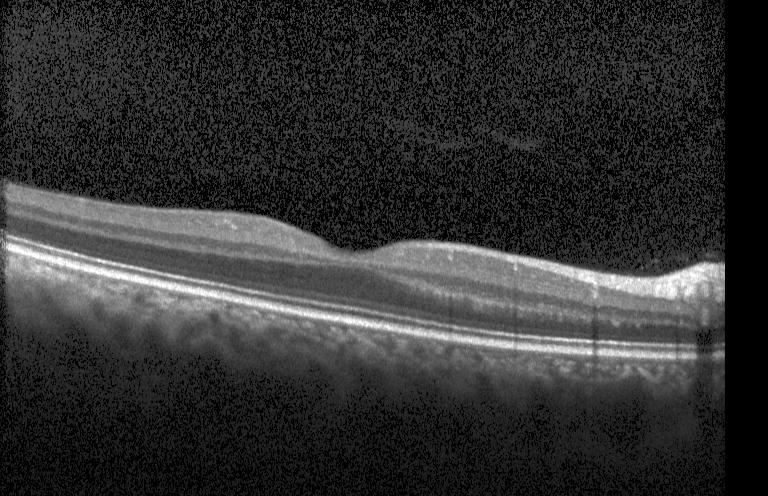
OCT line scan.
Impression: no evidence of CNV, DME, or drusen.